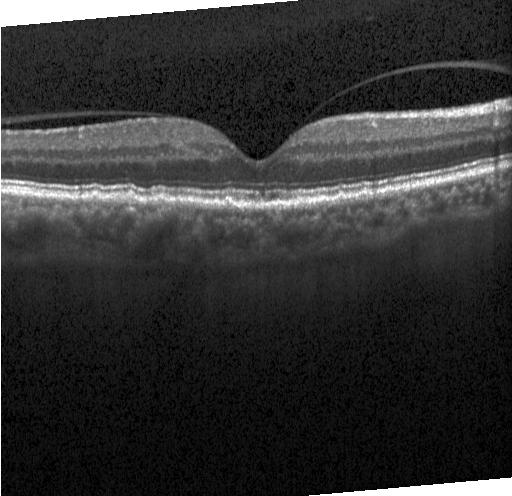

Optical coherence tomography B-scan.
Finding: drusen.